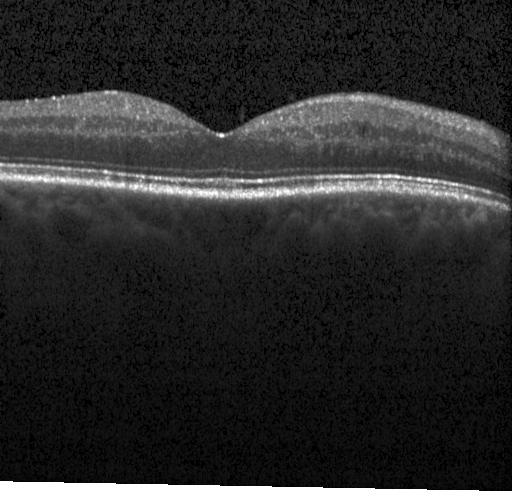
Optical coherence tomography B-scan. OCT finding: no choroidal neovascularization, no diabetic macular edema, and no drusen.